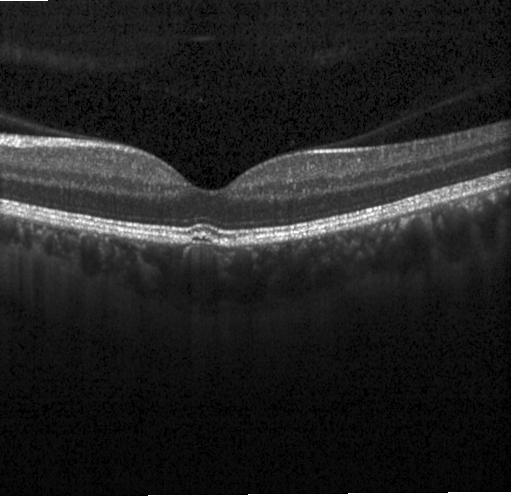
Centered on the fovea · spectral-domain optical coherence tomography · acquired on a Heidelberg Spectralis · retinal OCT B-scan
This B-scan demonstrates drusen.